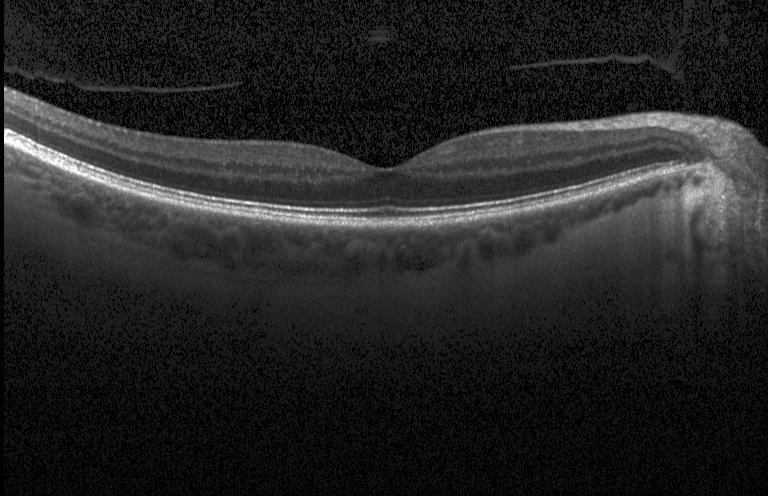

Dx: no evidence of choroidal neovascularization, diabetic macular edema, or drusen.